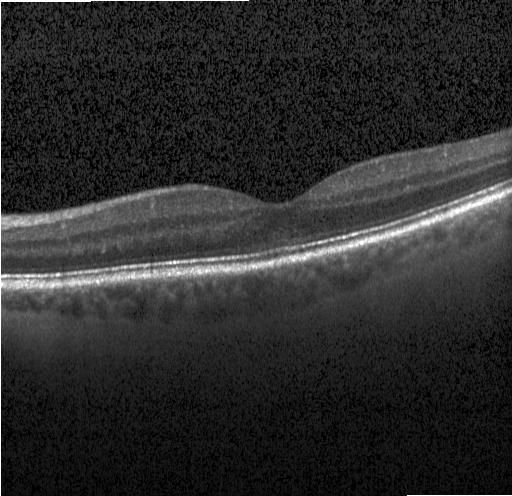

Neither CNV, DME, nor drusen.